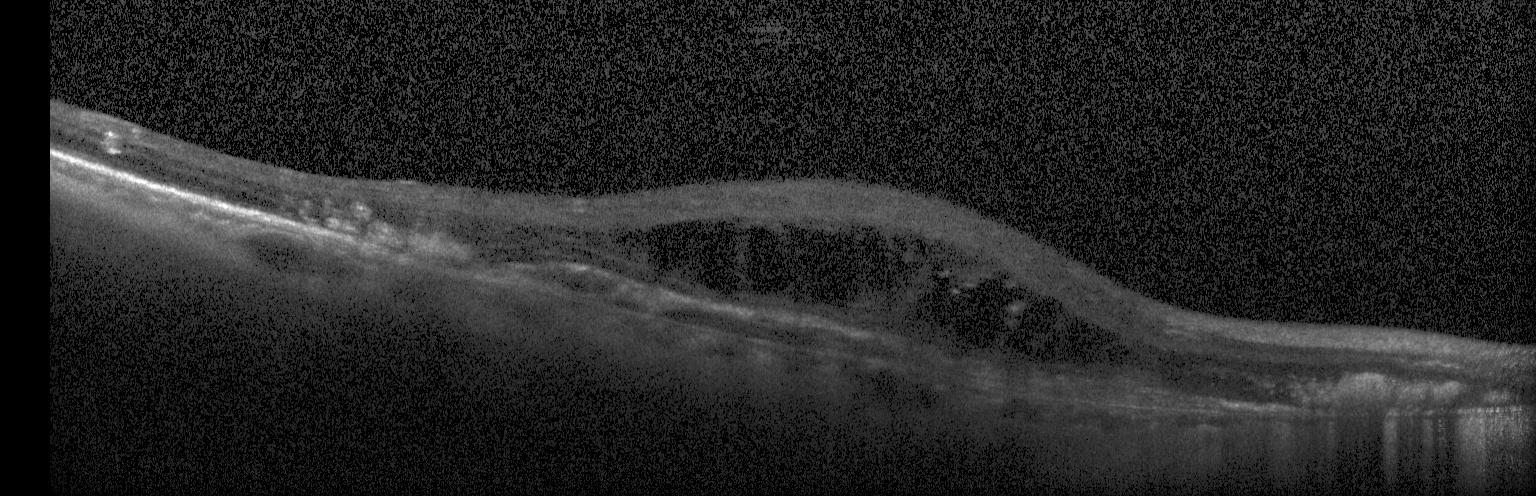 Spectral-domain OCT · OCT B-scan · acquired on a Heidelberg Spectralis · through the macula.
This B-scan demonstrates a choroidal neovascular membrane.